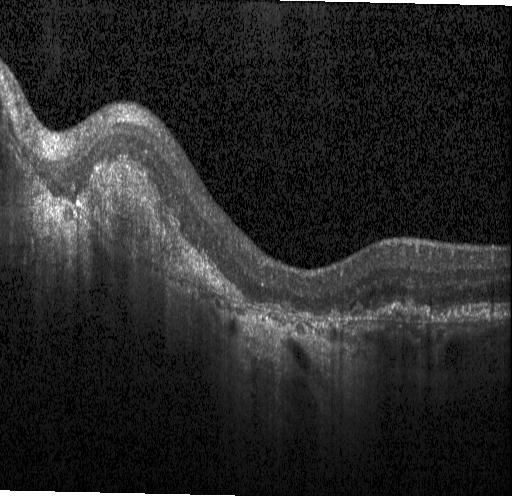 Retinal OCT cross-section
The scan shows choroidal neovascularization (CNV).